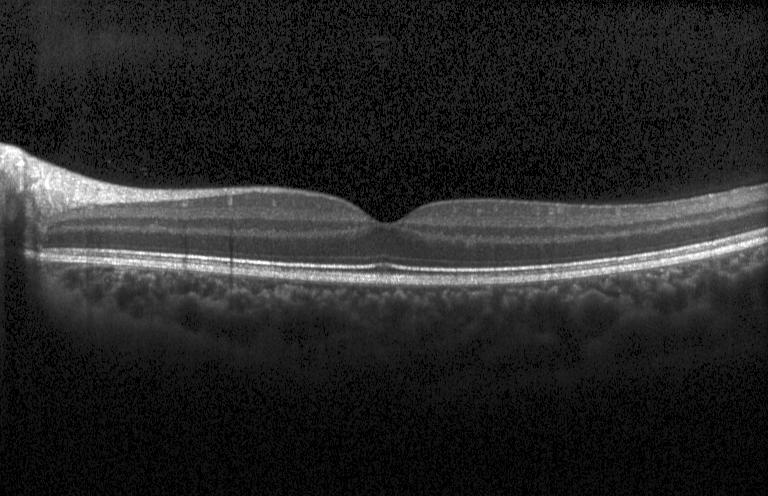

Finding: no CNV, DME, or drusen.